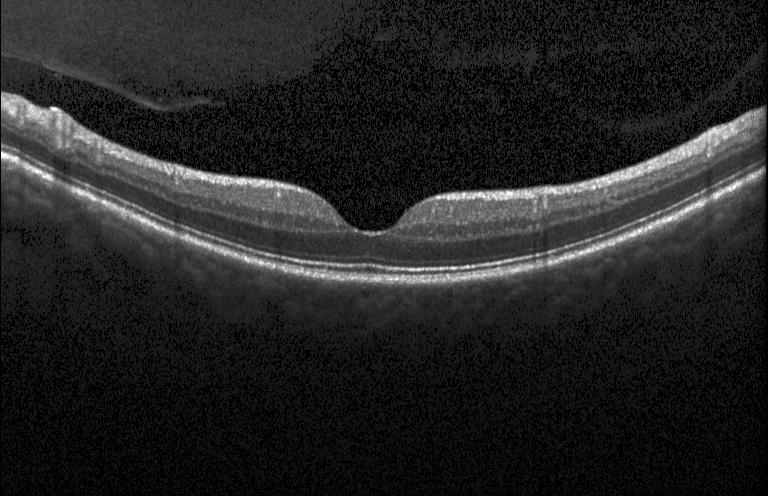

No choroidal neovascularization, diabetic macular edema, or drusen.